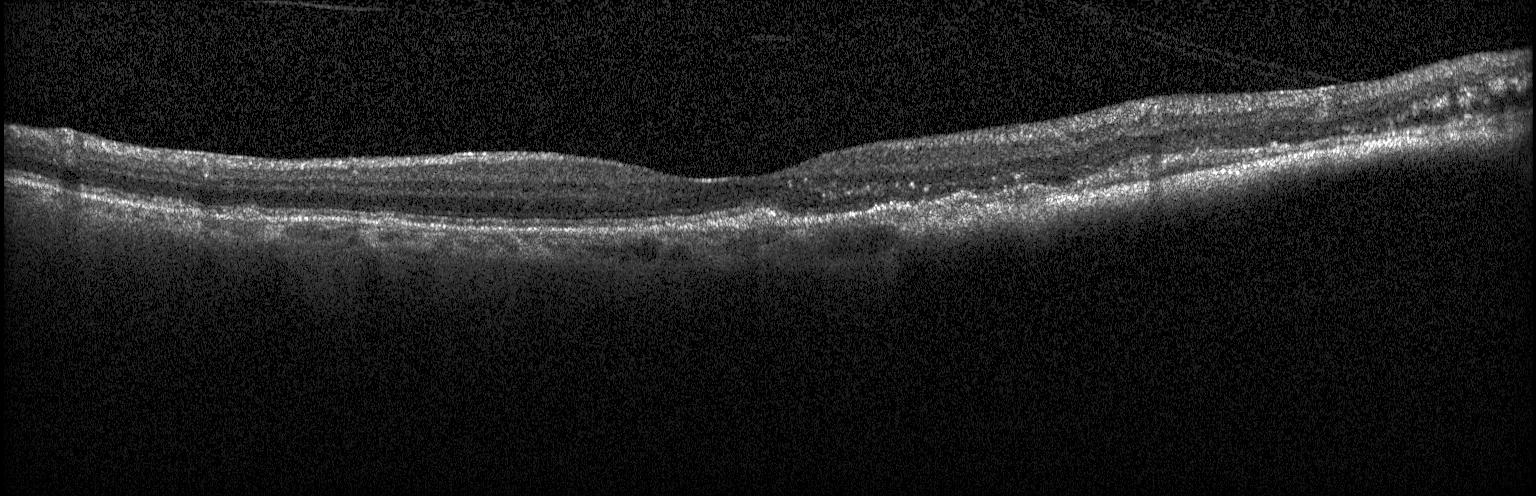 OCT B-scan.
Impression: a choroidal neovascular membrane.